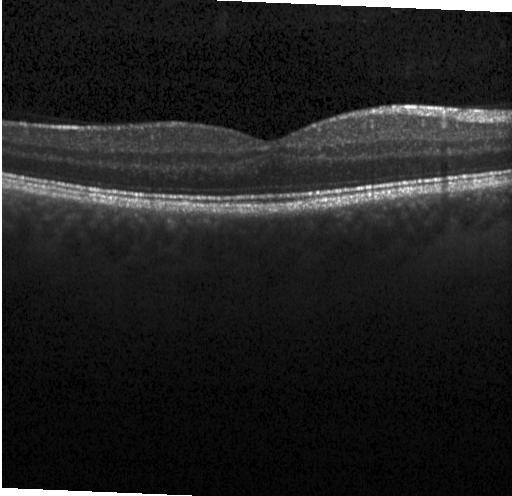
Finding: no evidence of choroidal neovascularization, diabetic macular edema, or drusen.